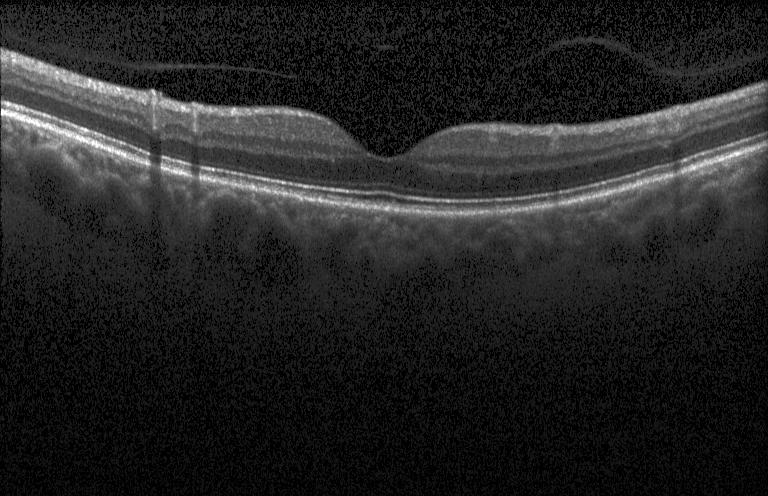
OCT finding: no choroidal neovascularization, diabetic macular edema, or drusen.